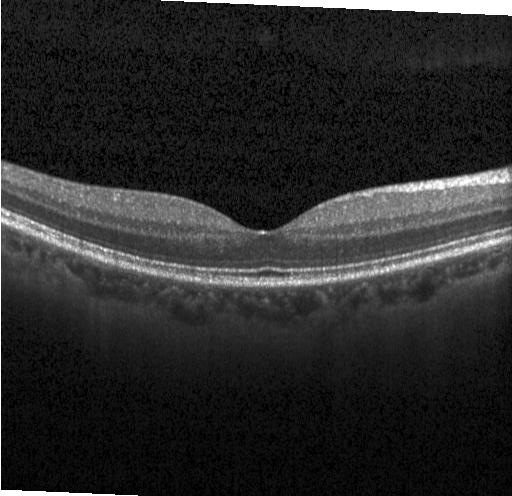 OCT line scan. Through the macula. Heidelberg Spectralis OCT system. Spectral-domain optical coherence tomography. This B-scan demonstrates no evidence of choroidal neovascularization, diabetic macular edema, or drusen.